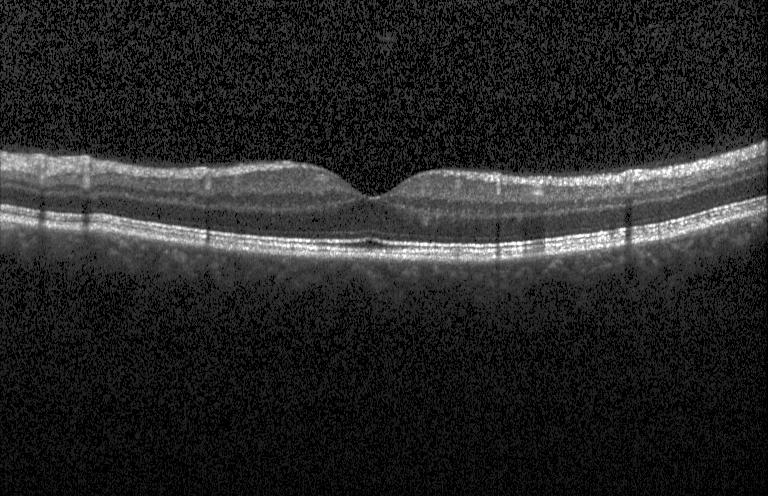 Retinal OCT B-scan, centered on the fovea, acquired on a Heidelberg Spectralis, SD-OCT.
Finding: no choroidal neovascularization, no diabetic macular edema, and no drusen.